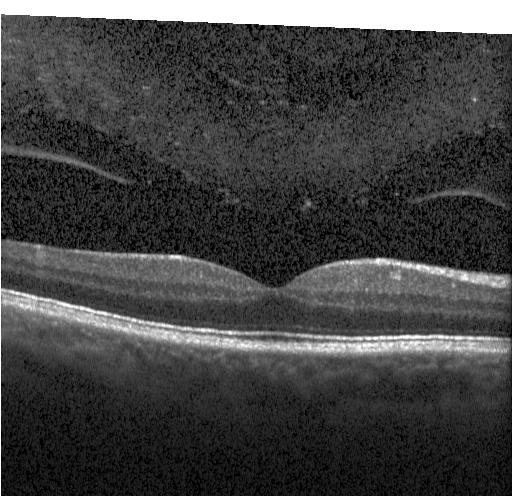
Acquired on a Heidelberg Spectralis, fovea-centered, spectral-domain OCT, optical coherence tomography scan — Impression: no evidence of CNV, DME, or drusen.